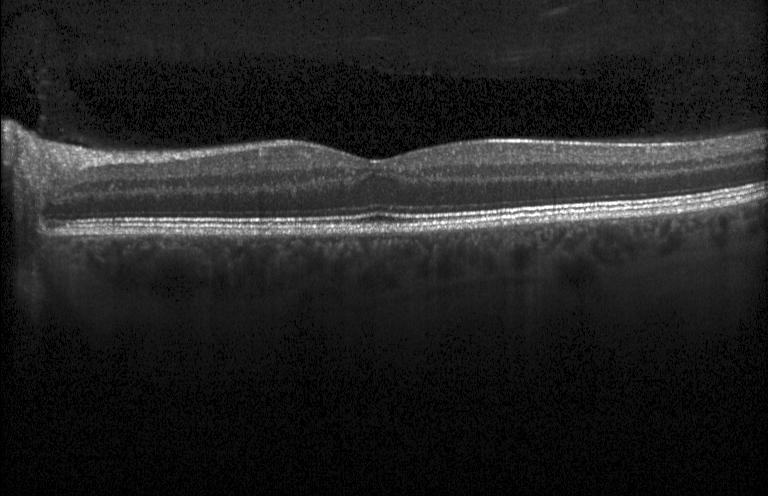 Finding: neither choroidal neovascularization, diabetic macular edema, nor drusen.